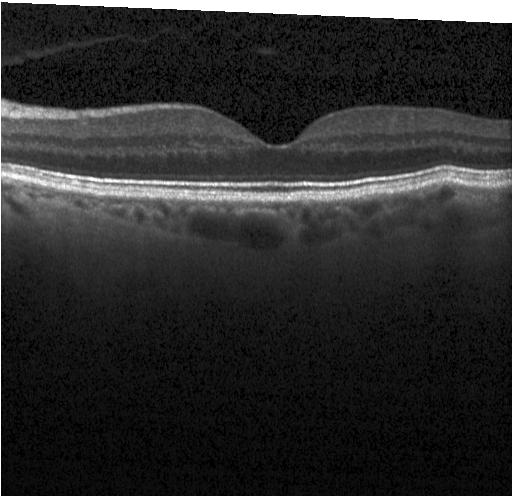 Fovea-centered; optical coherence tomography scan. Impression: no evidence of CNV, DME, or drusen.